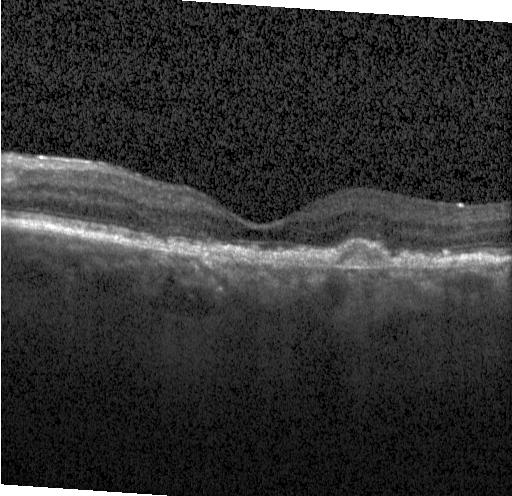

Finding: a choroidal neovascular membrane.